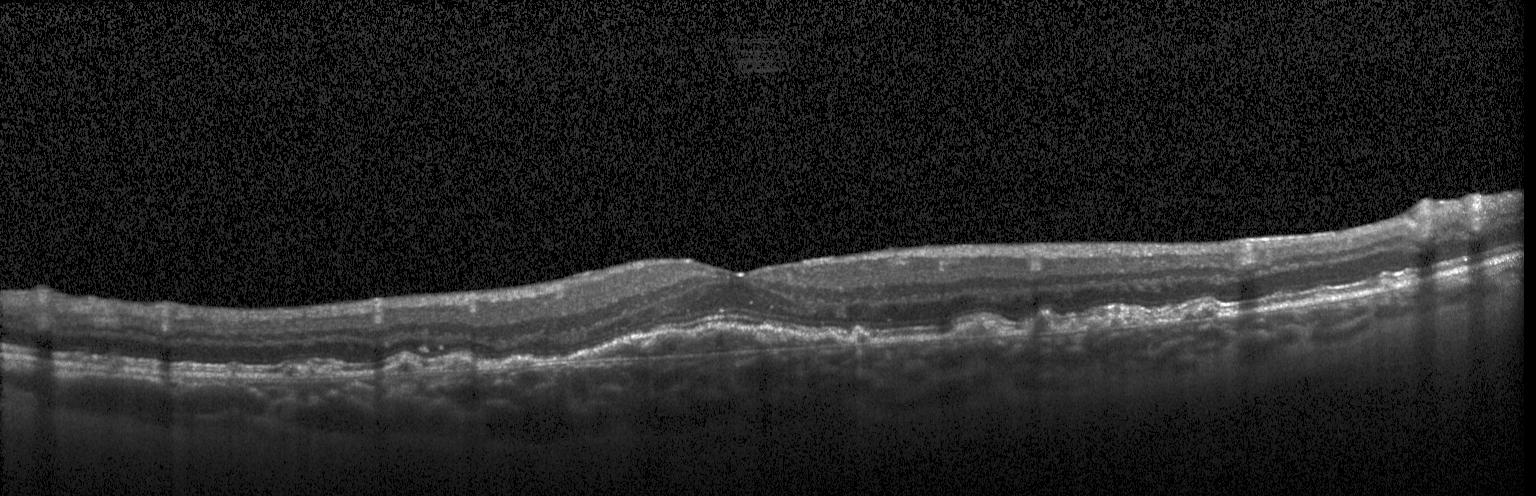 Fovea-centered; retinal OCT B-scan — Macular OCT: choroidal neovascularization (CNV).